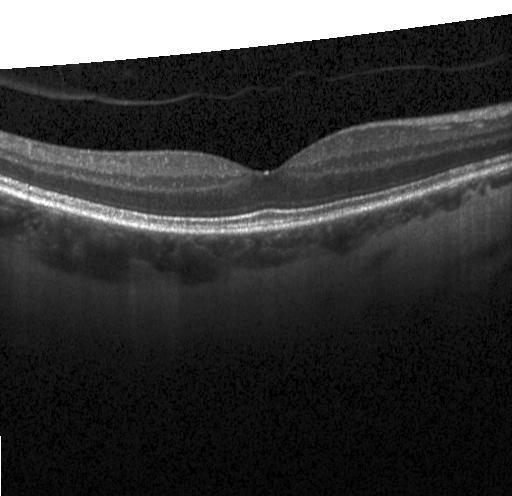
OCT B-scan · Heidelberg Spectralis OCT system · spectral-domain OCT — OCT finding: no CNV, no DME, and no drusen.